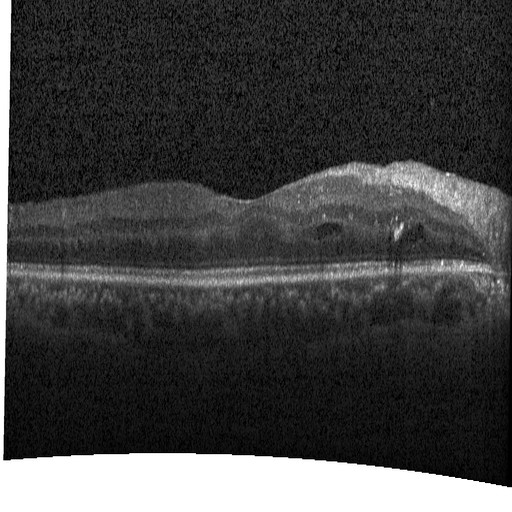

Diabetic macular edema (DME).